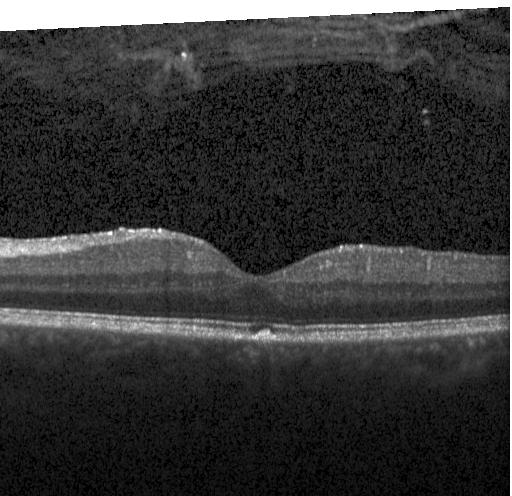
Finding: drusen.